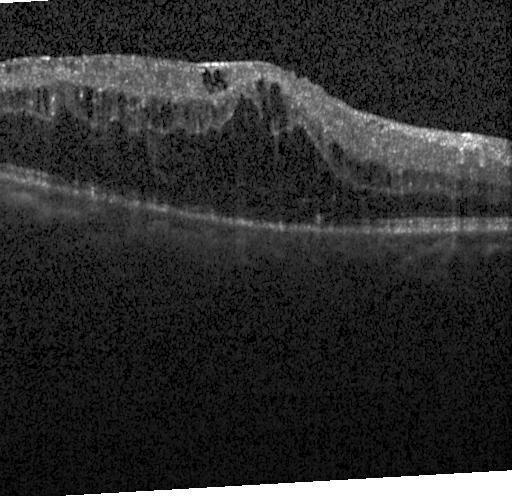
This B-scan demonstrates diabetic macular edema (DME).